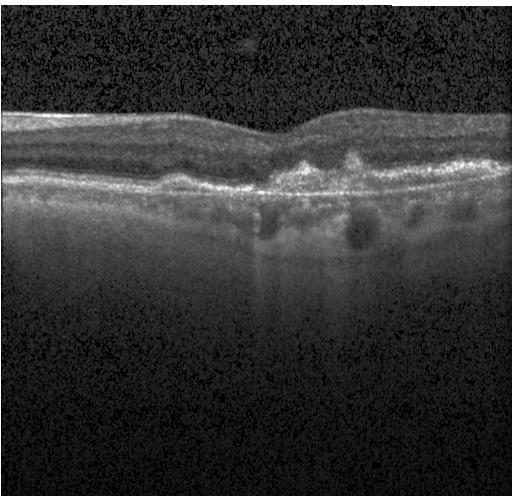

Acquired on a Heidelberg Spectralis, OCT line scan
Macular OCT: a choroidal neovascular membrane.